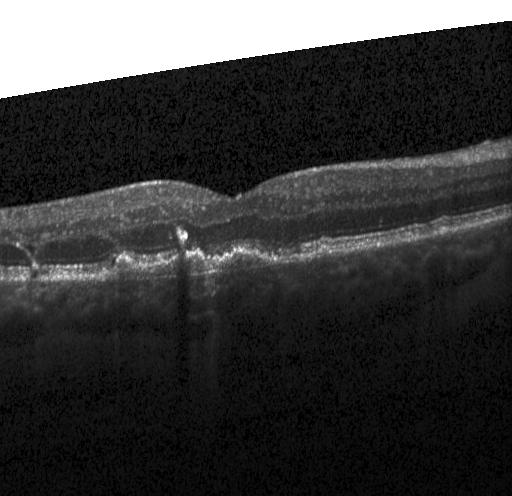 Acquired on a Heidelberg Spectralis. Optical coherence tomography B-scan. Spectral-domain OCT. Fovea-centered.
This B-scan demonstrates a choroidal neovascular membrane.